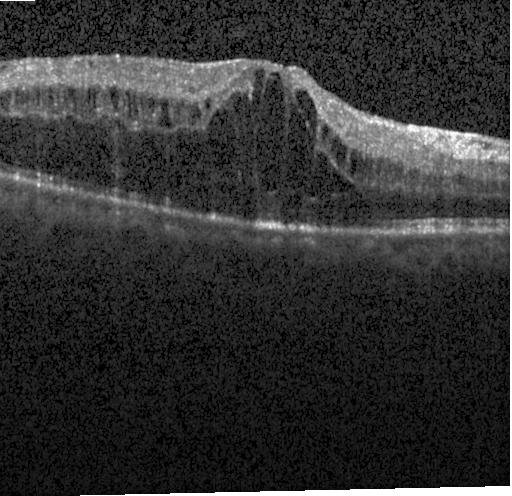

Spectral-domain OCT B-scan: diabetic macular edema.